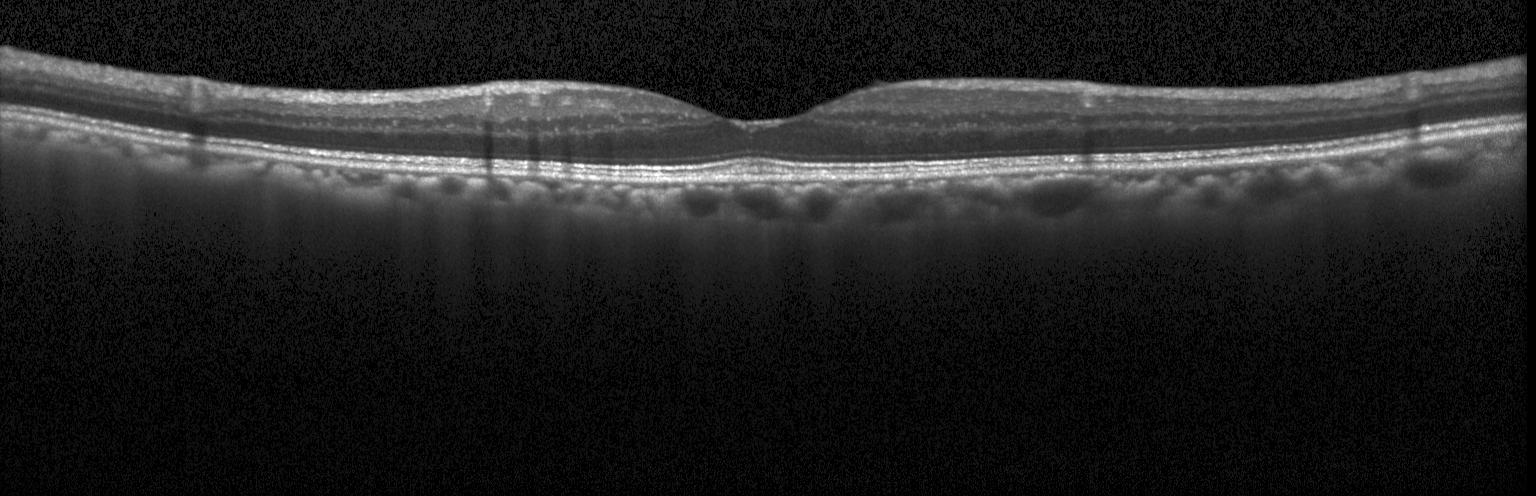 Heidelberg Spectralis OCT system, SD-OCT, centered on the fovea, OCT B-scan. Impression: neither choroidal neovascularization, diabetic macular edema, nor drusen.